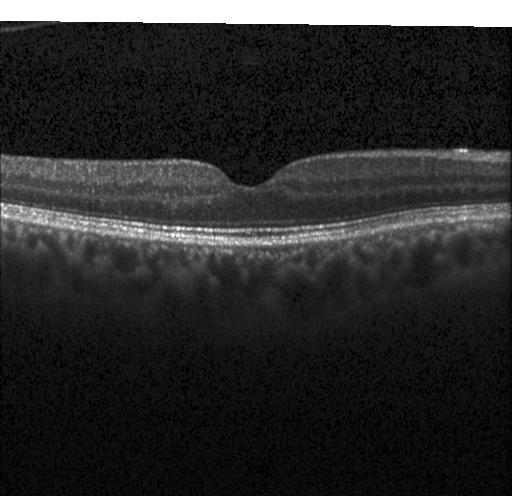 OCT finding: no evidence of choroidal neovascularization, diabetic macular edema, or drusen.